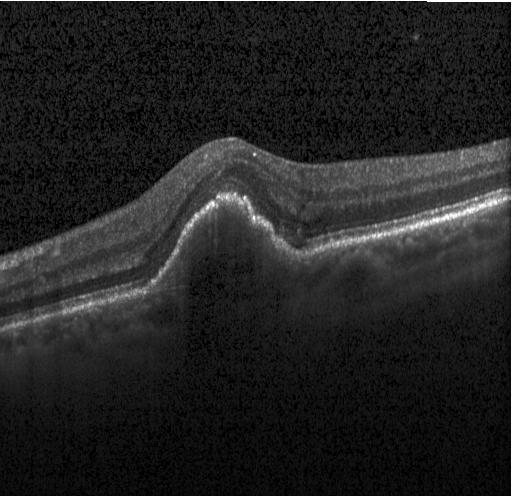

Finding: CNV.